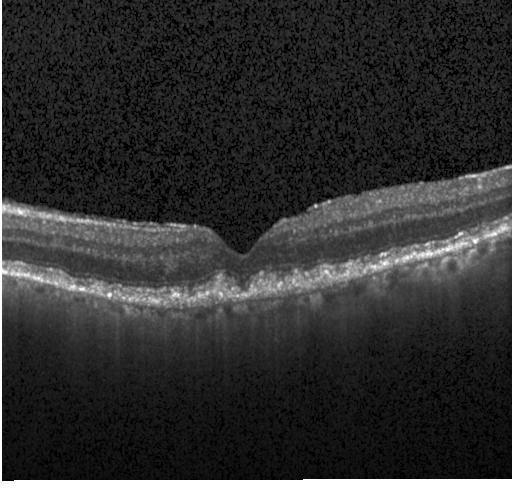
Assessment: sub-RPE drusenoid deposits.